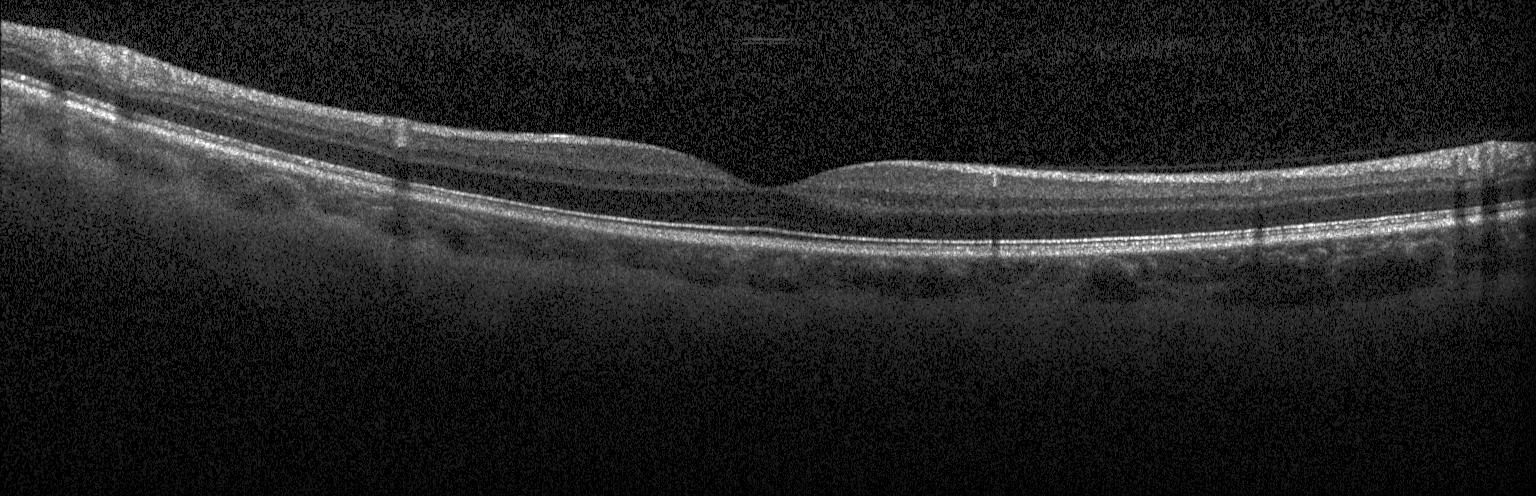

Optical coherence tomography B-scan · Heidelberg Spectralis.
The scan shows no choroidal neovascularization, no diabetic macular edema, and no drusen.